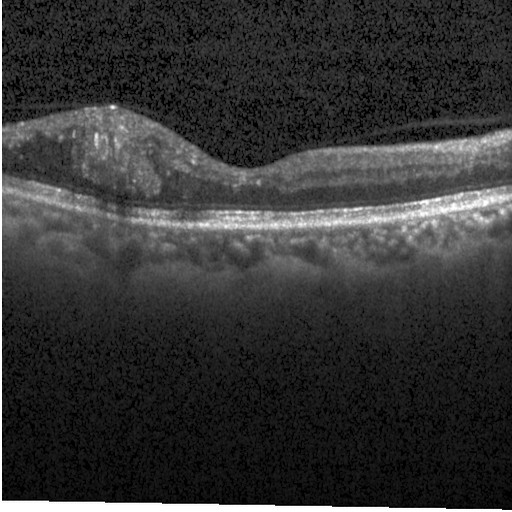

Acquired on a Heidelberg Spectralis, horizontal scan through the fovea, optical coherence tomography B-scan
Finding: DME.